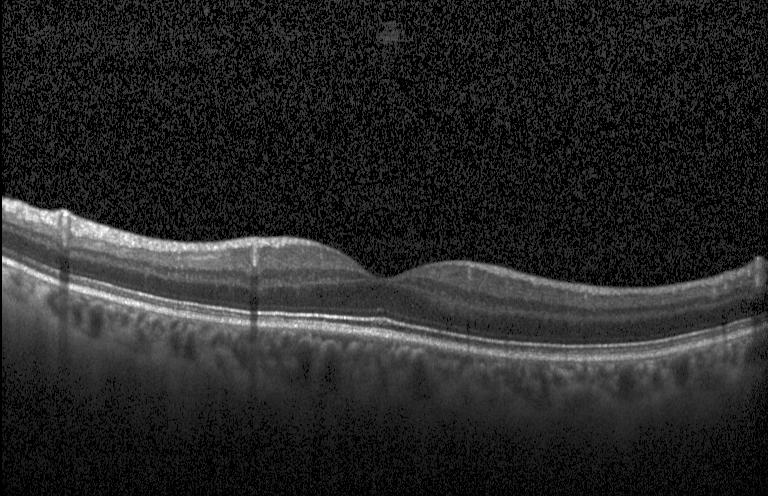
Optical coherence tomography scan — The scan shows no evidence of choroidal neovascularization, diabetic macular edema, or drusen.